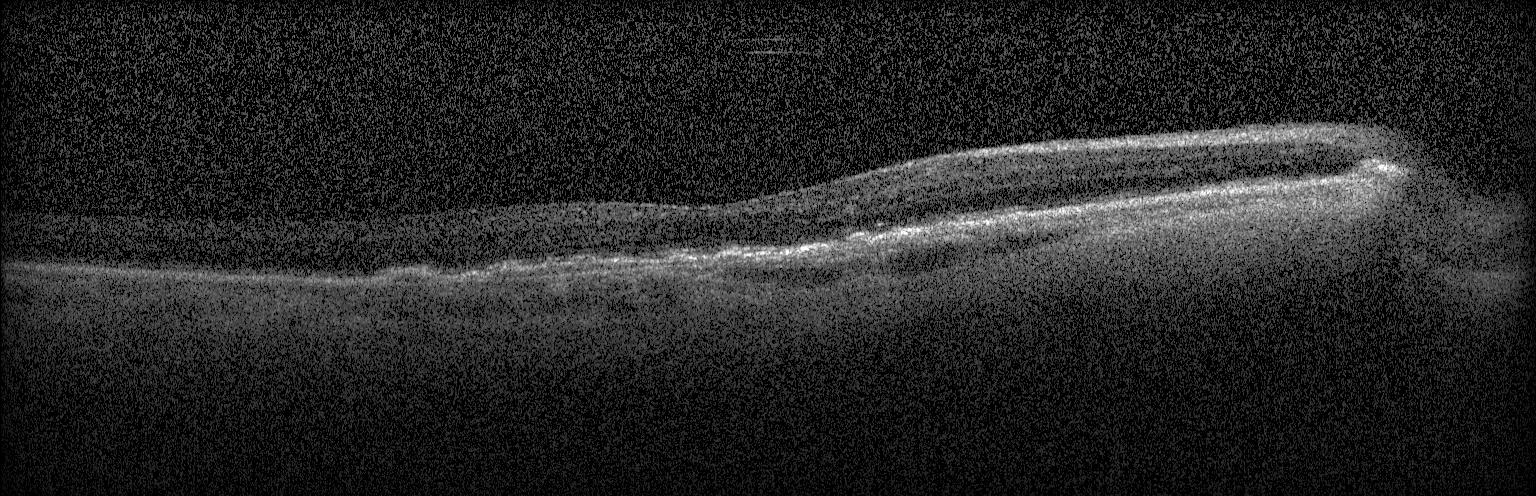

Dx: choroidal neovascularization (CNV).